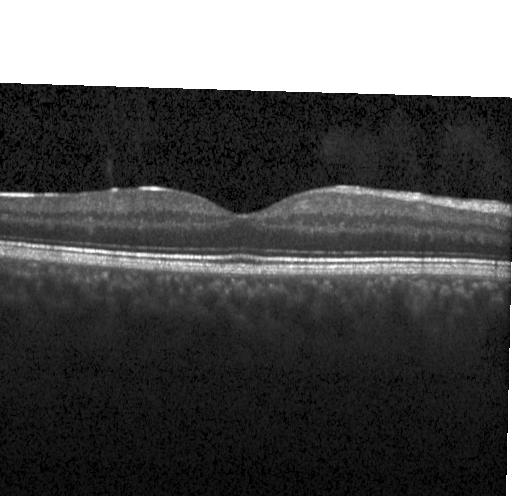

Retinal OCT cross-section showing neither choroidal neovascularization, diabetic macular edema, nor drusen.